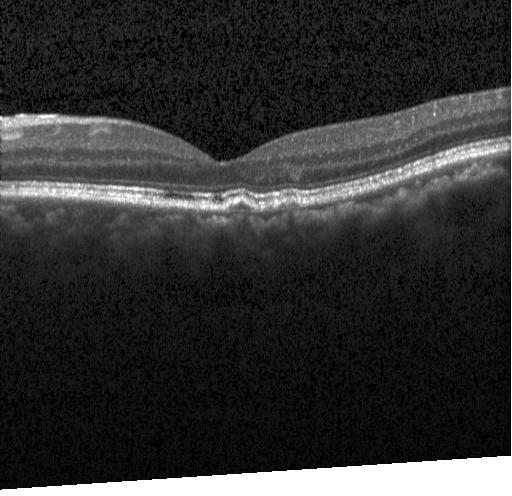

Finding: drusen.